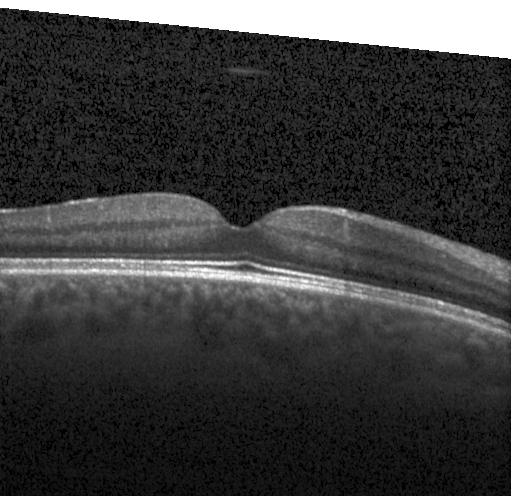 Heidelberg Spectralis OCT system, OCT B-scan, SD-OCT, fovea-centered
The scan shows no CNV, no DME, and no drusen.